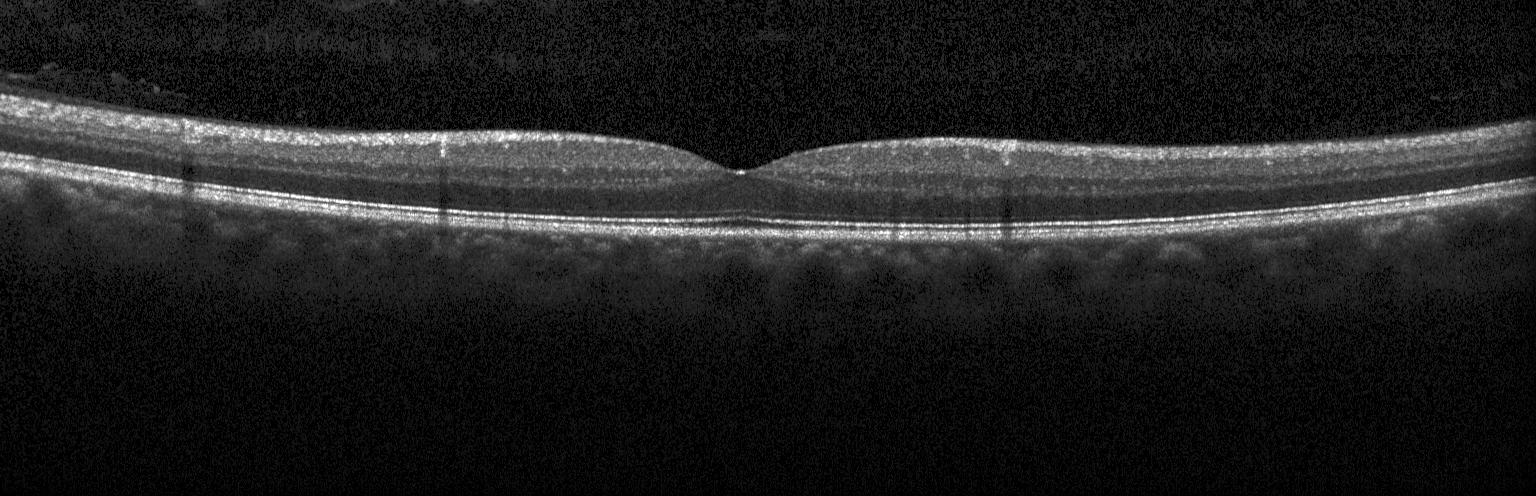 Heidelberg Spectralis; centered on the fovea; retinal OCT cross-section; SD-OCT. Finding: neither CNV, DME, nor drusen.